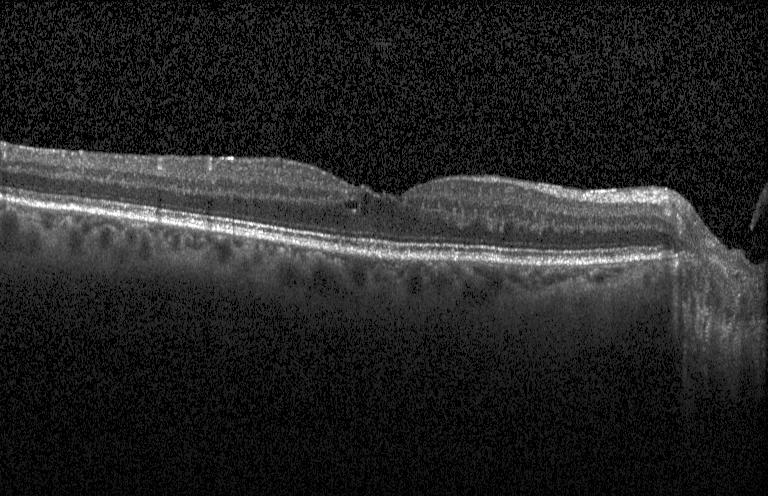 Retinal OCT B-scan; centered on the fovea; spectral-domain optical coherence tomography.
Impression: DME.